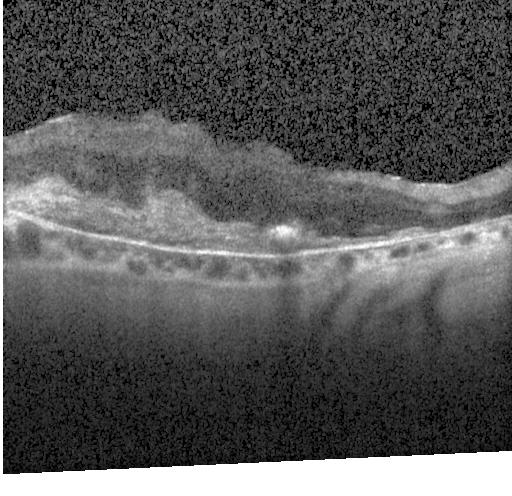

OCT B-scan.
This B-scan demonstrates choroidal neovascularization (CNV).